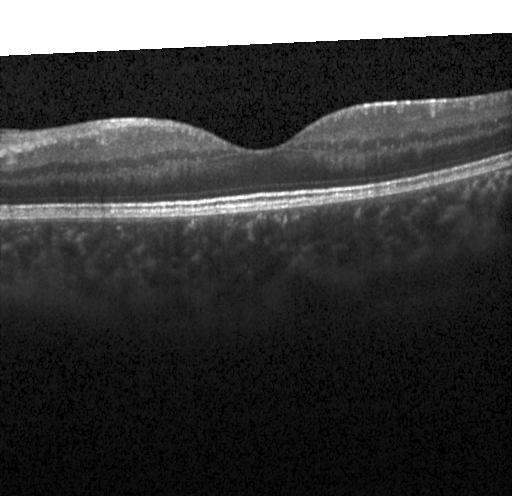

This B-scan demonstrates neither choroidal neovascularization, diabetic macular edema, nor drusen.